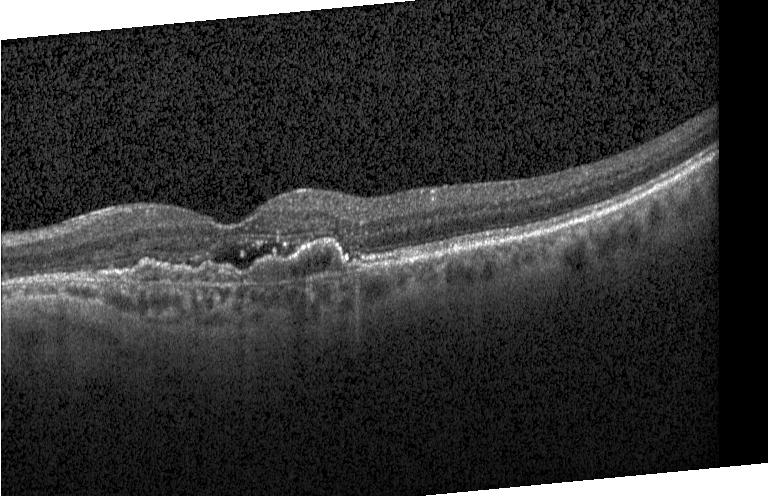

Retinal OCT cross-section.
OCT finding: choroidal neovascularization.